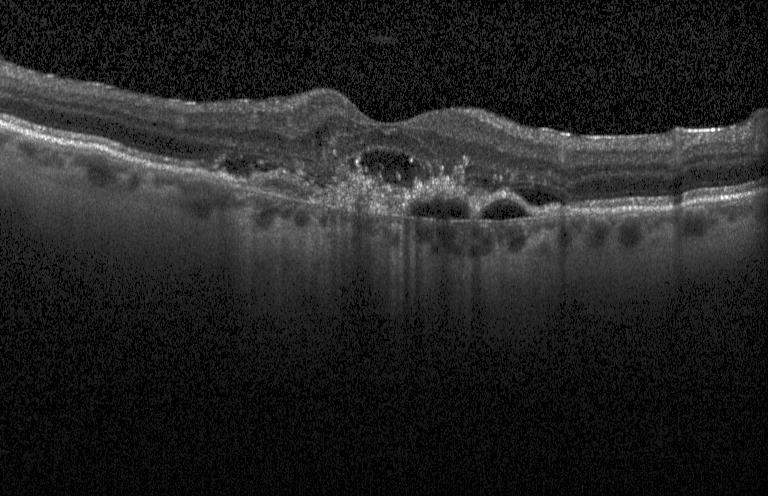
Finding: a choroidal neovascular membrane.